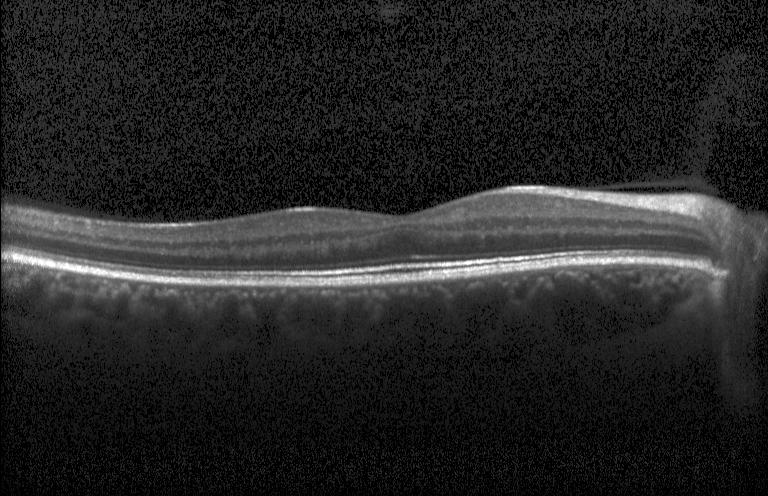 Retinal OCT B-scan. Impression: no choroidal neovascularization, no diabetic macular edema, and no drusen.